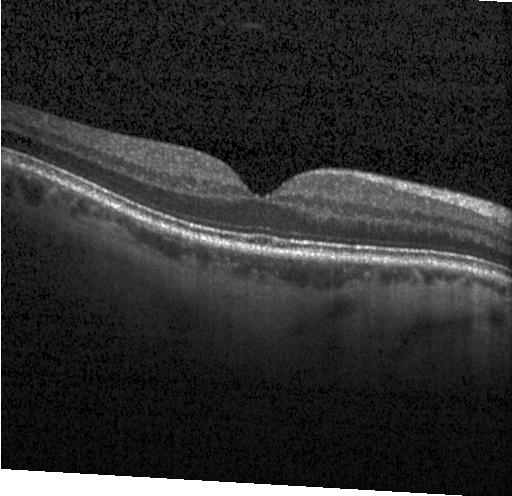

The scan shows neither choroidal neovascularization, diabetic macular edema, nor drusen.